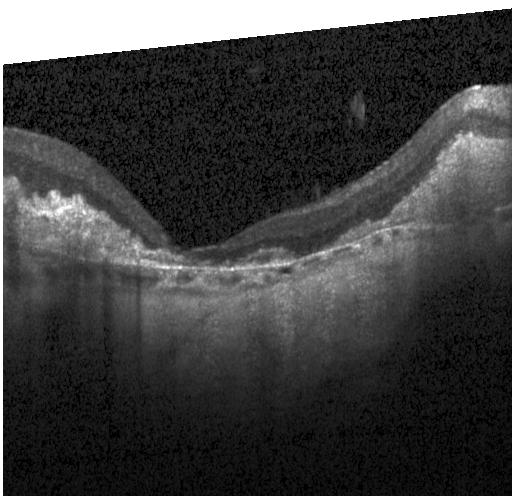 Macular scan; SD-OCT; optical coherence tomography scan; Heidelberg Spectralis OCT system. Dx: choroidal neovascularization.